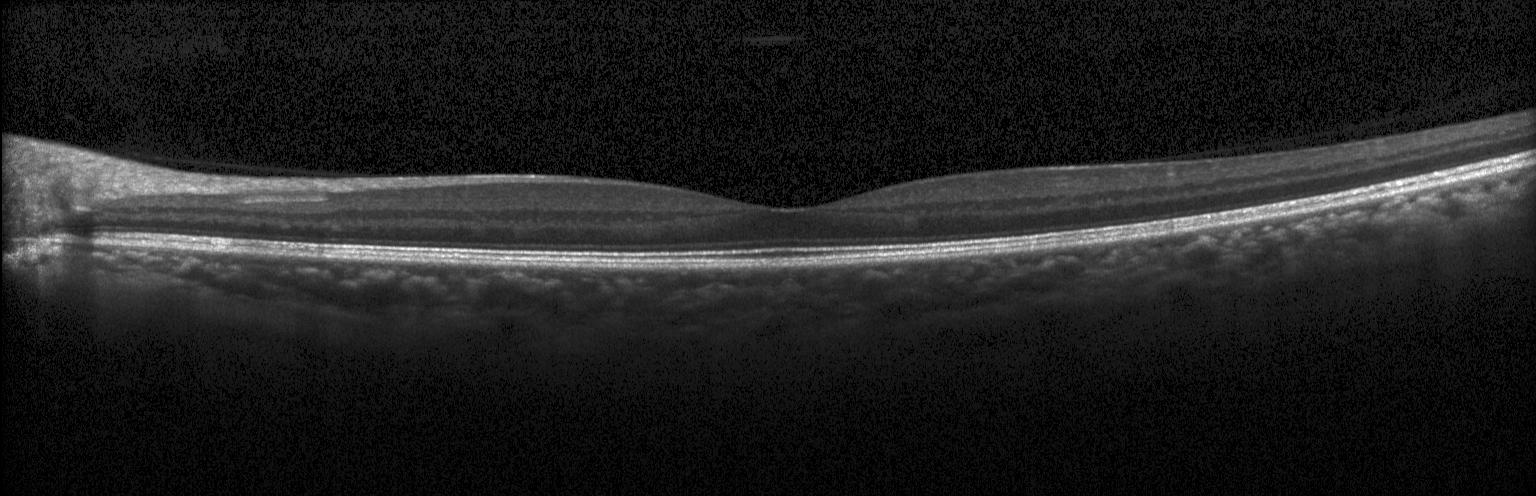
Diagnosis: no evidence of CNV, DME, or drusen.